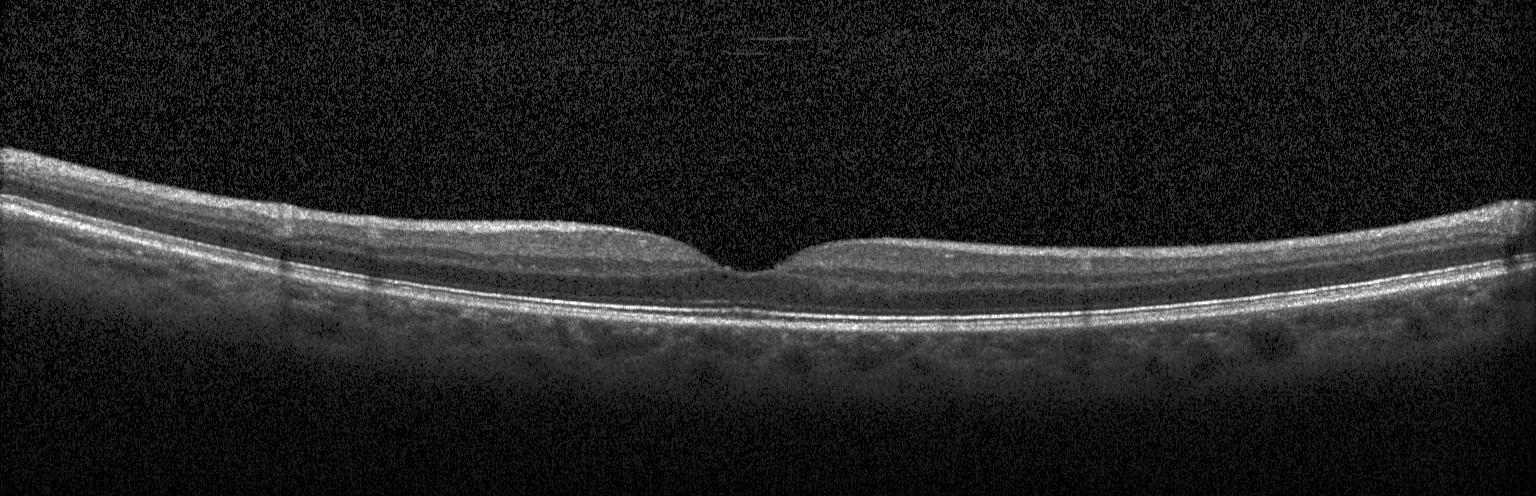
OCT scan showing neither choroidal neovascularization, diabetic macular edema, nor drusen.